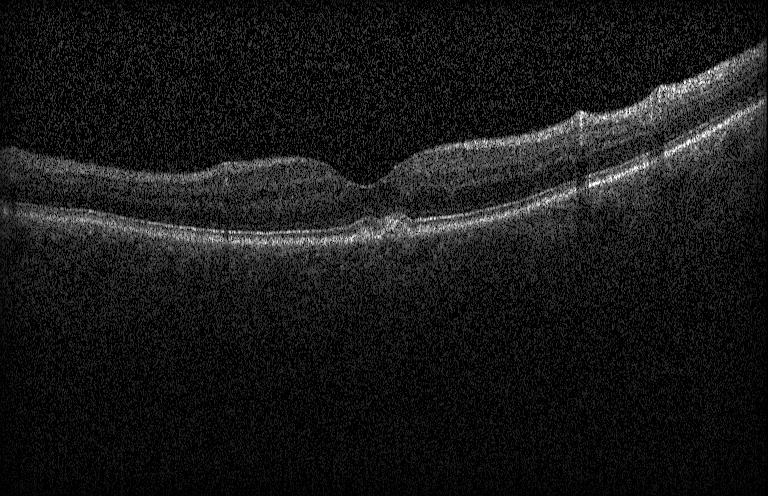
Centered on the fovea · spectral-domain OCT · OCT line scan · Heidelberg Spectralis. Finding: sub-RPE drusenoid deposits.